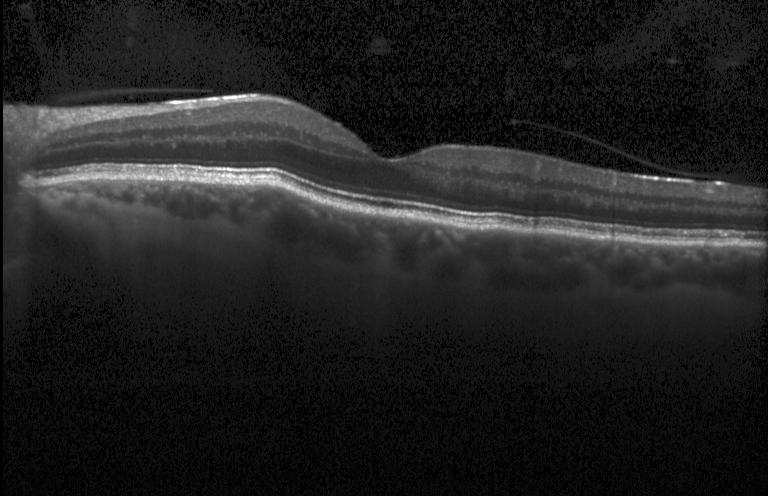
Retinal OCT B-scan
Macular OCT: no choroidal neovascularization, diabetic macular edema, or drusen.